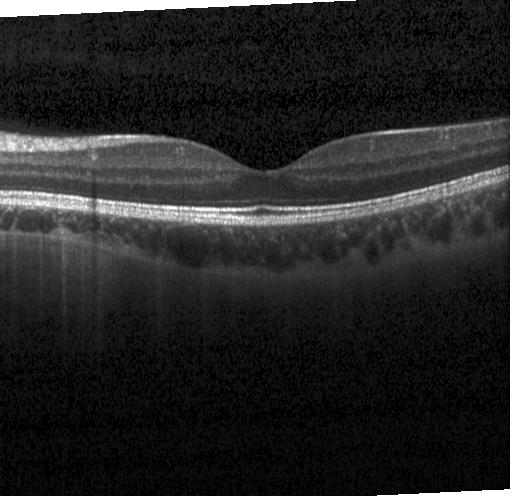 Macular OCT: no choroidal neovascularization, no diabetic macular edema, and no drusen.